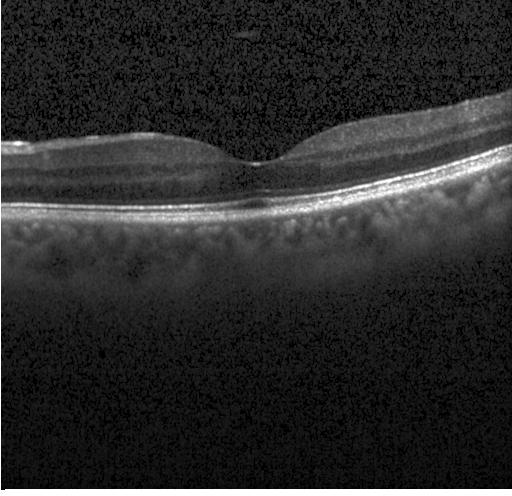
OCT B-scan, spectral-domain optical coherence tomography, Heidelberg Spectralis, through the macula — Diagnosis: neither choroidal neovascularization, diabetic macular edema, nor drusen.